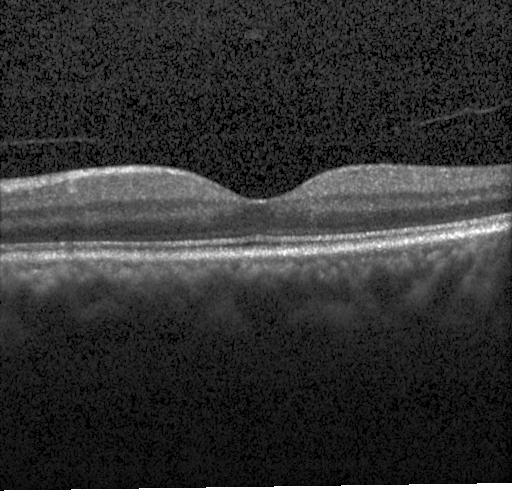

OCT B-scan. Diagnosis: no choroidal neovascularization, no diabetic macular edema, and no drusen.